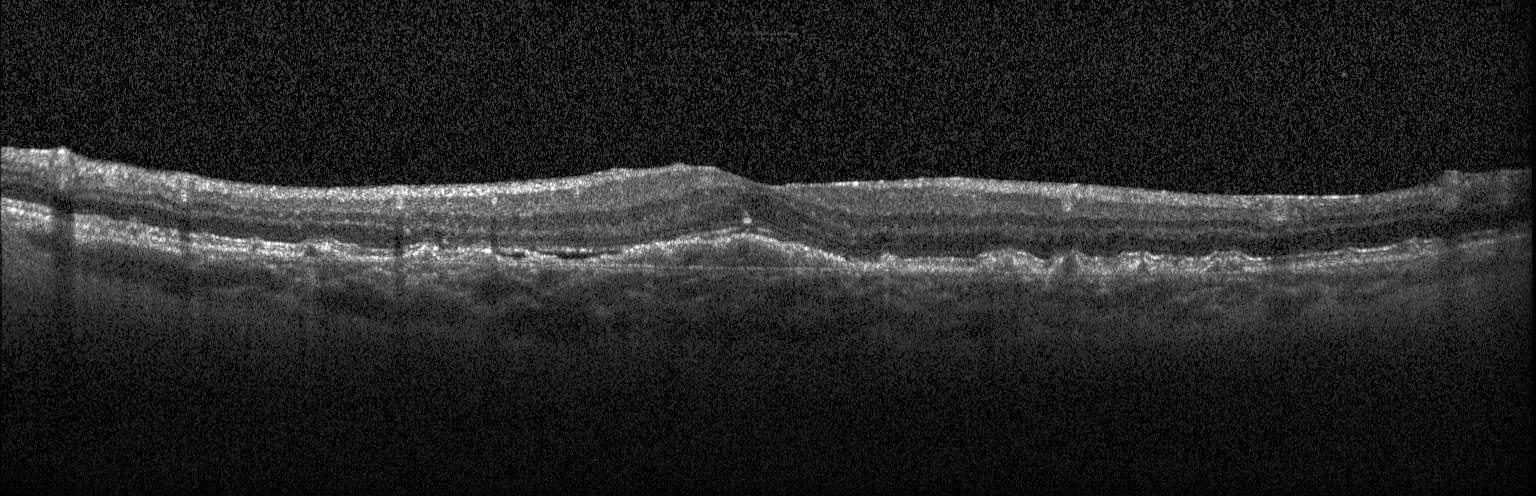

Fovea-centered; retinal OCT cross-section
Finding: a choroidal neovascular membrane.